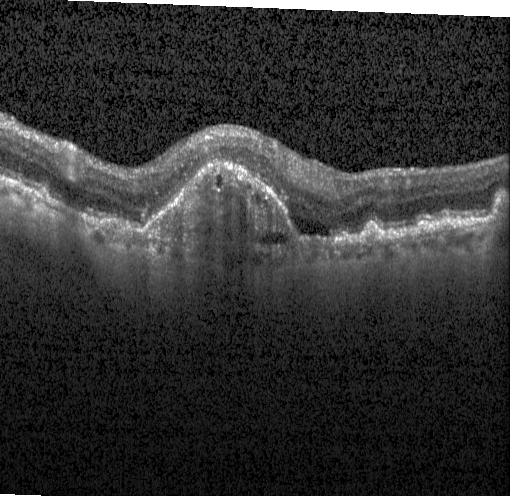

OCT B-scan. Acquired on a Heidelberg Spectralis. Spectral-domain OCT. Through the macula.
A choroidal neovascular membrane.